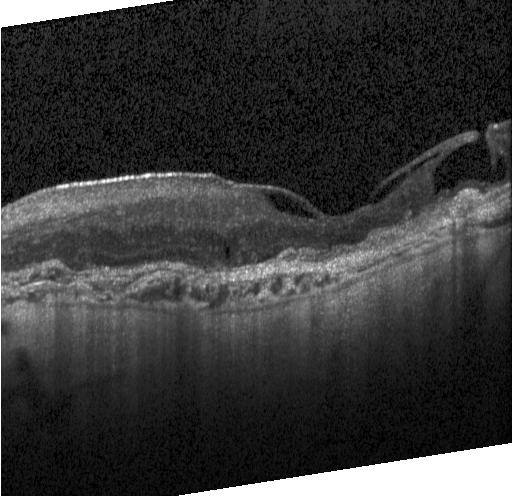

Optical coherence tomography scan. Horizontal scan through the fovea. SD-OCT.
Impression: CNV.